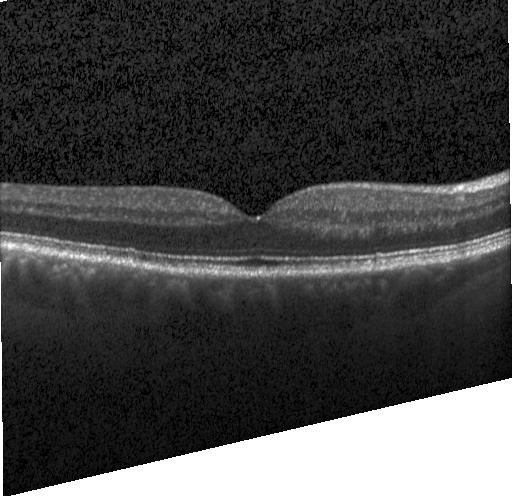

SD-OCT · horizontal scan through the fovea · Heidelberg Spectralis OCT system · retinal OCT B-scan. The scan shows no evidence of choroidal neovascularization, diabetic macular edema, or drusen.